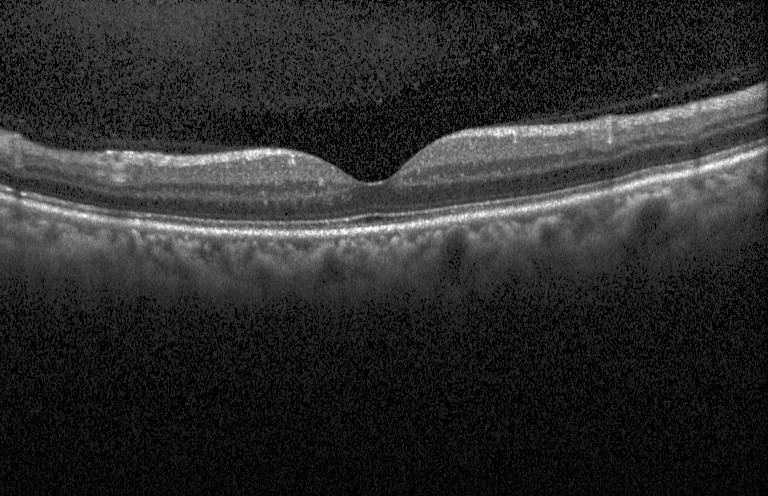

Diagnosis: neither CNV, DME, nor drusen.